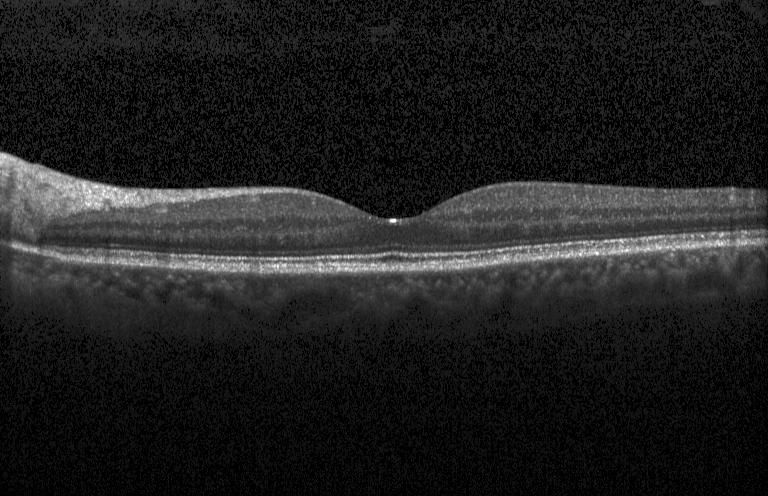

OCT line scan. Spectral-domain OCT
The scan shows no CNV, no DME, and no drusen.